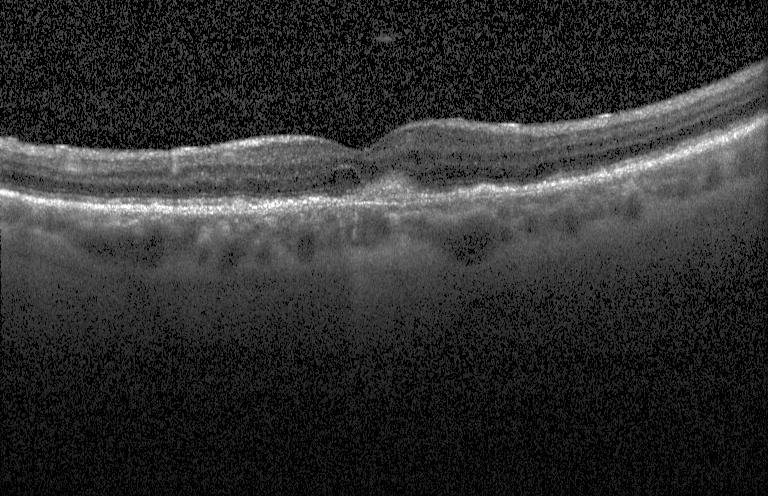

Centered on the fovea; retinal OCT cross-section; Heidelberg Spectralis OCT system.
The scan shows a choroidal neovascular membrane.